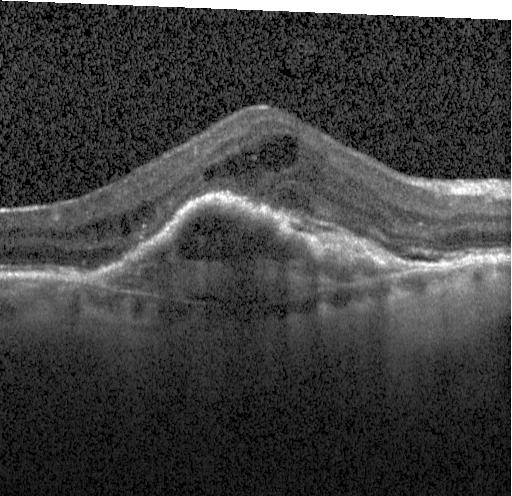

Retinal OCT B-scan.
Impression: a choroidal neovascular membrane.